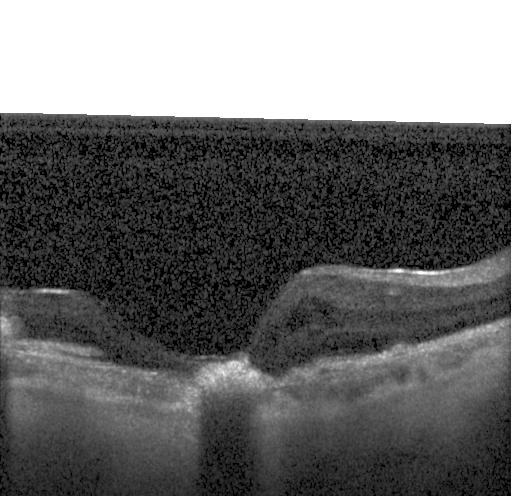 Retinal OCT B-scan — Macular OCT: a choroidal neovascular membrane.